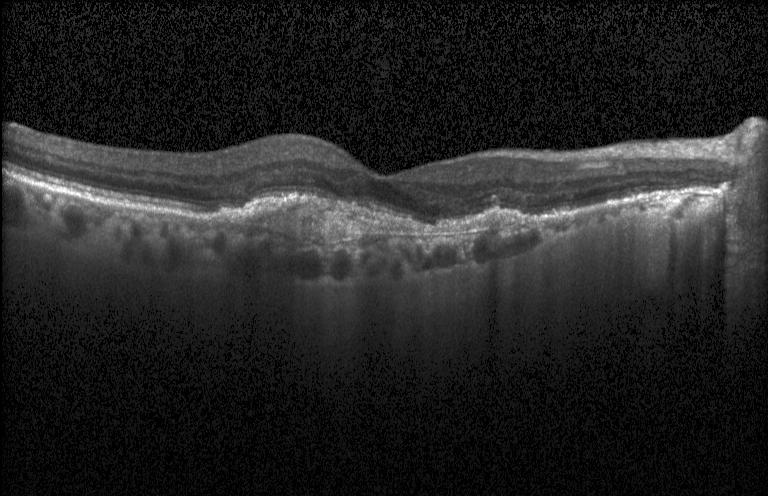 OCT B-scan, fovea-centered, acquired on a Heidelberg Spectralis, spectral-domain optical coherence tomography. OCT finding: CNV.